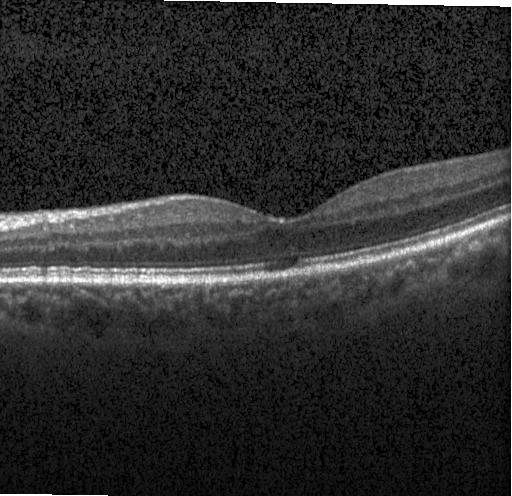
Spectral-domain OCT · OCT B-scan
Impression: no evidence of choroidal neovascularization, diabetic macular edema, or drusen.